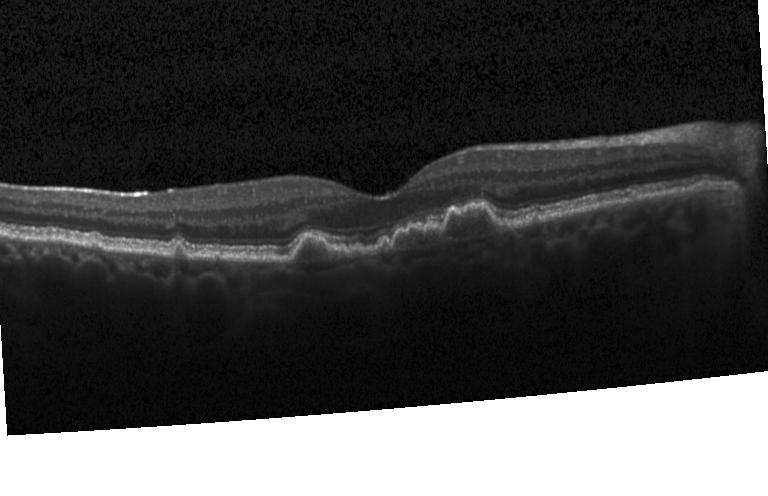
Dx: drusen.